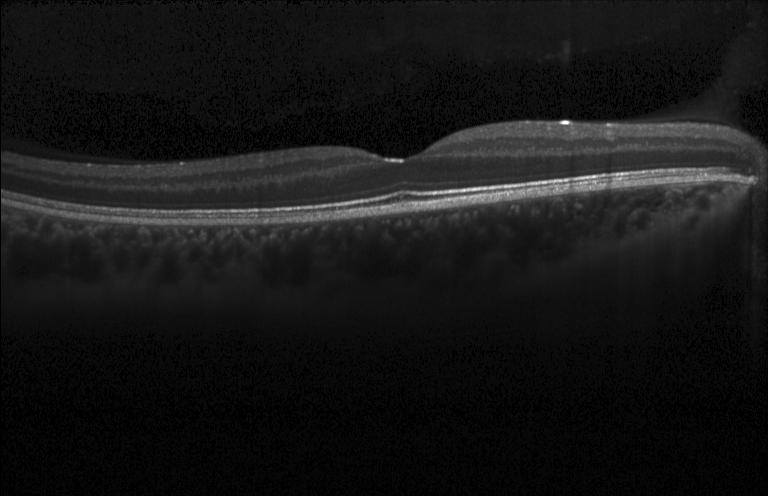 Dx: no evidence of CNV, DME, or drusen.